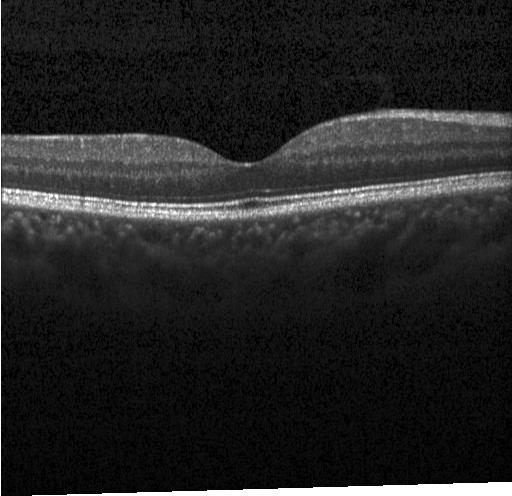

Heidelberg Spectralis OCT system · optical coherence tomography B-scan. Impression: no CNV, no DME, and no drusen.